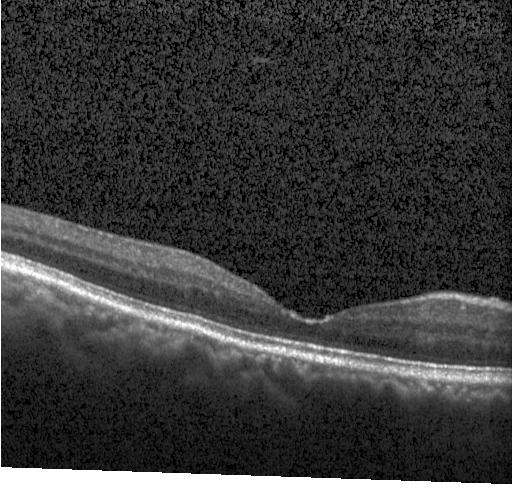 Horizontal scan through the fovea, optical coherence tomography B-scan, spectral-domain optical coherence tomography, Heidelberg Spectralis
Impression: no evidence of choroidal neovascularization, diabetic macular edema, or drusen.